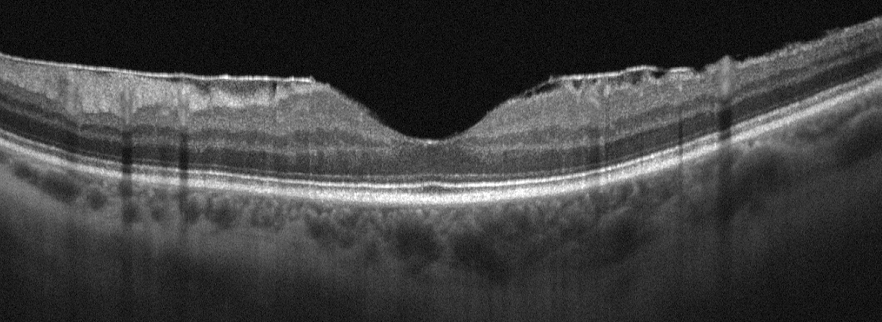

Impression: epiretinal membrane (ERM).